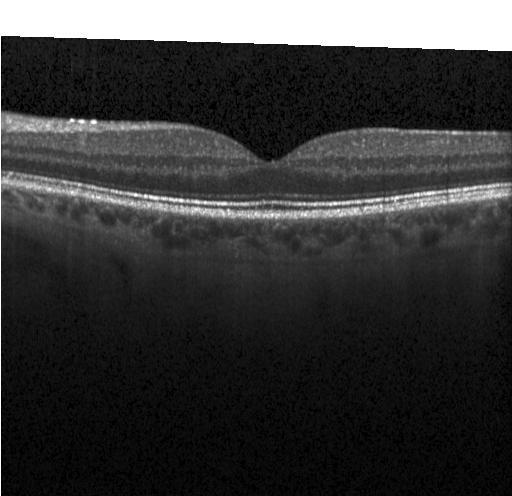

OCT line scan, horizontal scan through the fovea. The scan shows no evidence of choroidal neovascularization, diabetic macular edema, or drusen.